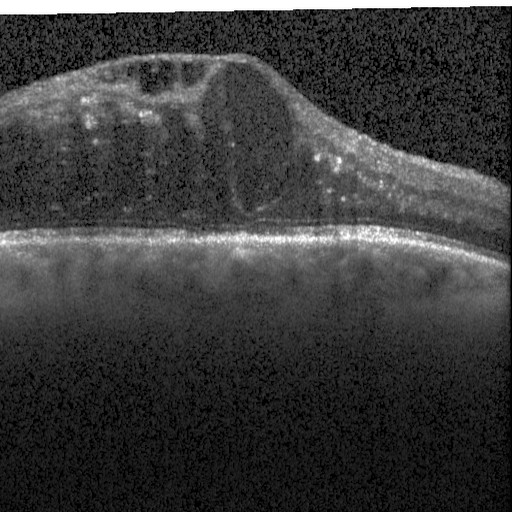 Impression: diabetic macular edema (DME).